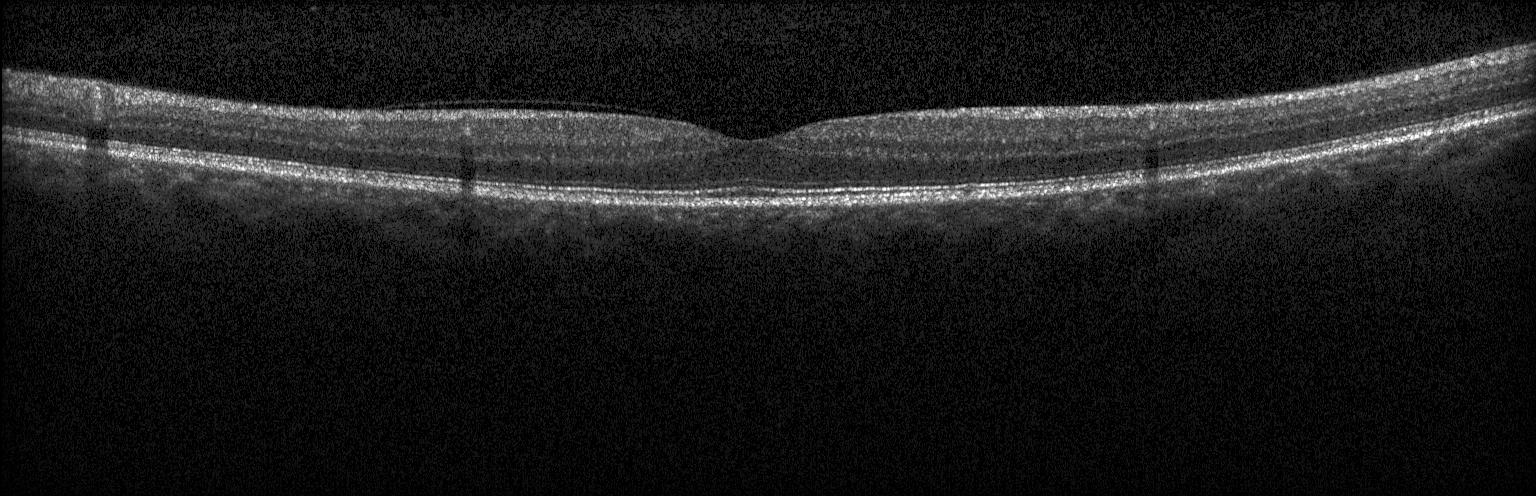 Optical coherence tomography B-scan. Acquired on a Heidelberg Spectralis
OCT finding: neither choroidal neovascularization, diabetic macular edema, nor drusen.